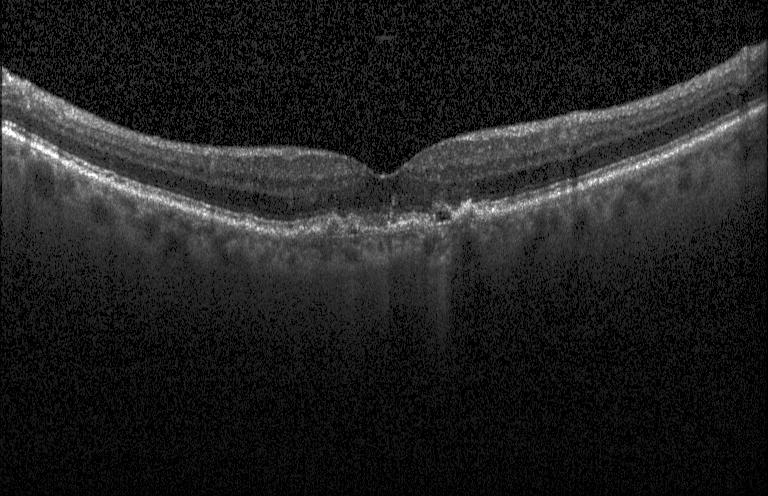

A choroidal neovascular membrane.